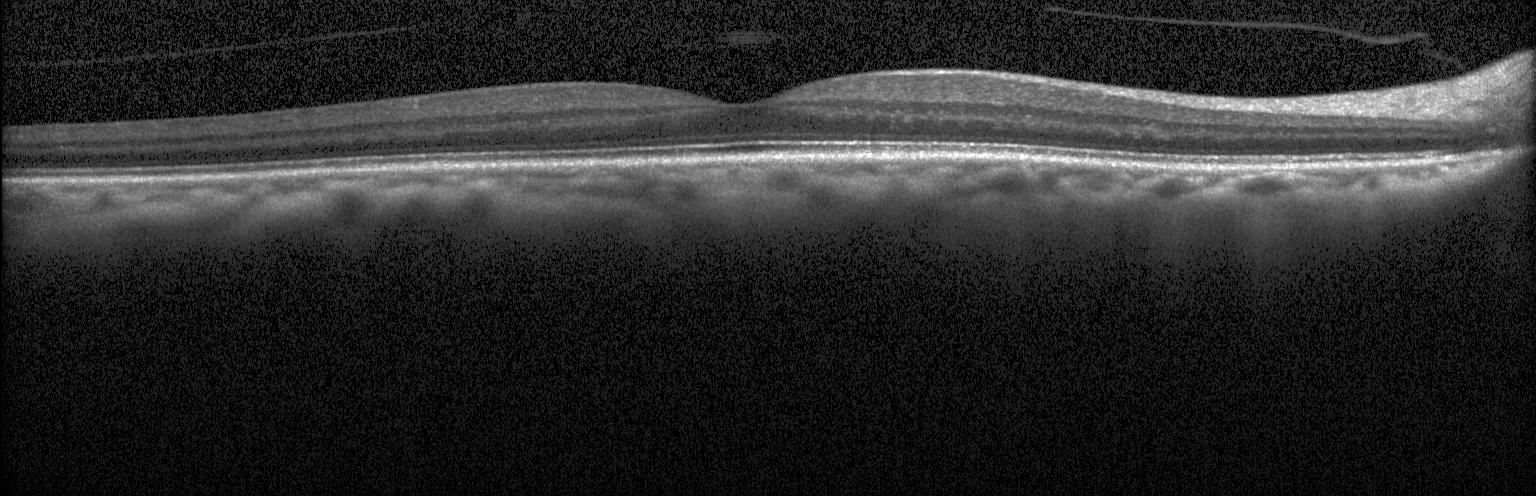
Horizontal scan through the fovea, spectral-domain OCT, instrument: Heidelberg Spectralis, retinal OCT cross-section. Diagnosis: no choroidal neovascularization, no diabetic macular edema, and no drusen.